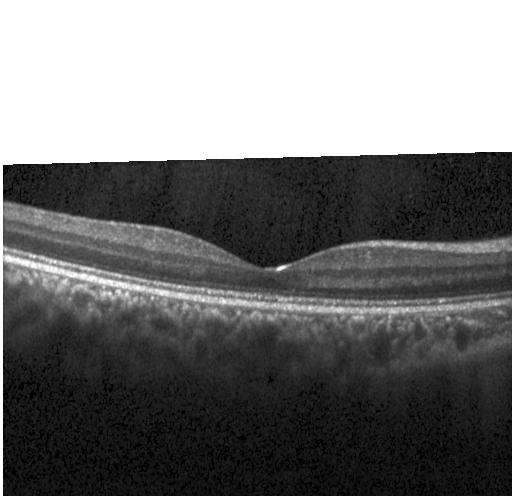 Retinal OCT B-scan, instrument: Heidelberg Spectralis, centered on the fovea, SD-OCT.
Dx: no CNV, no DME, and no drusen.